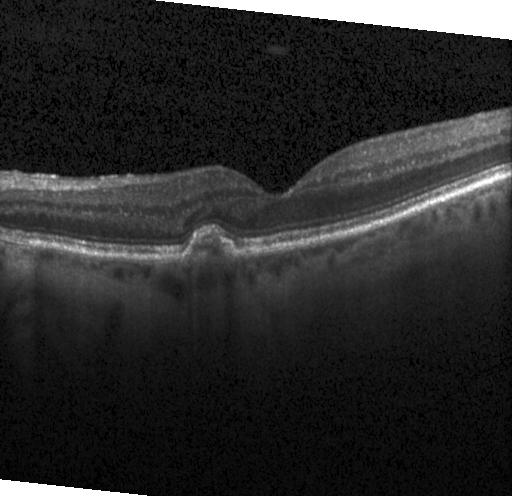 Acquired on a Heidelberg Spectralis, optical coherence tomography scan. Macular OCT: a choroidal neovascular membrane.